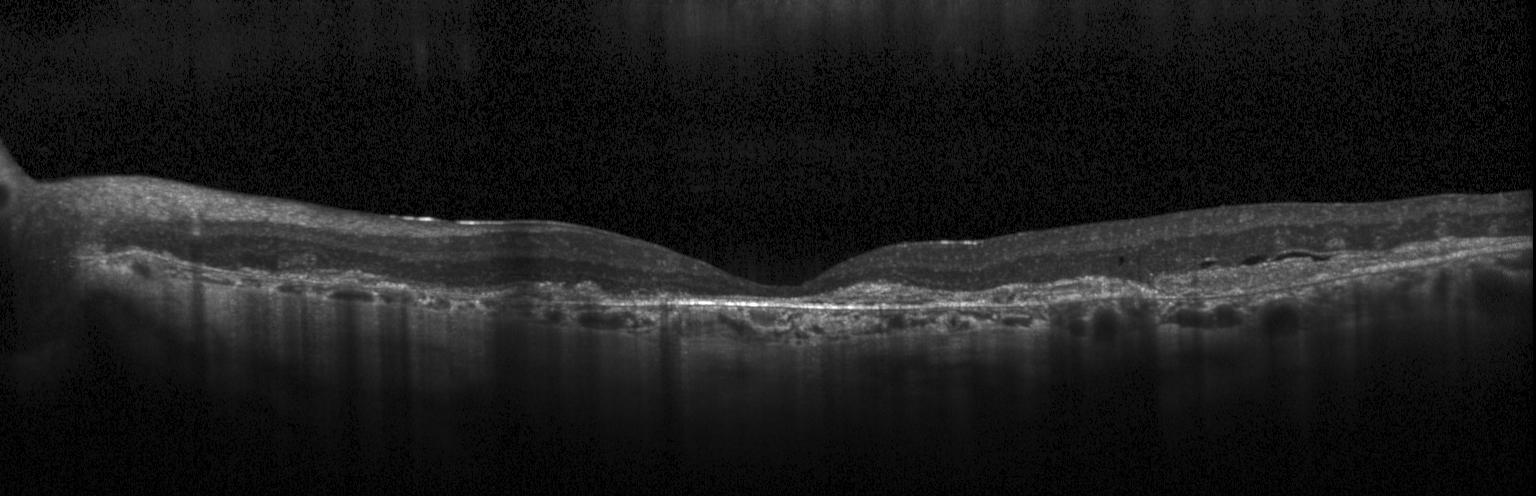
Finding: CNV.